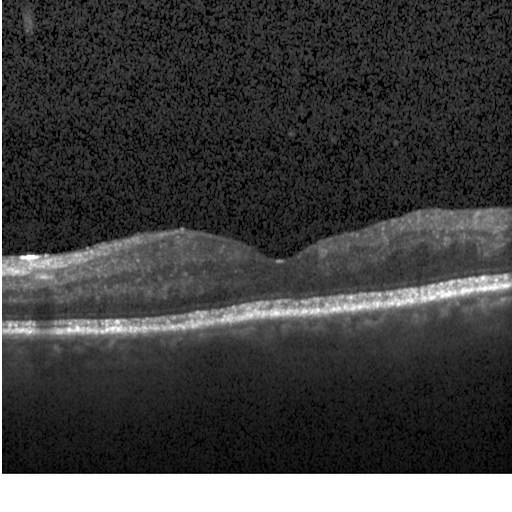

This B-scan demonstrates DME.